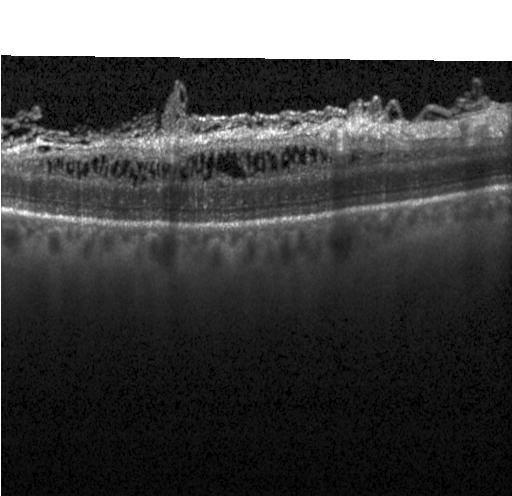 Retinal OCT cross-section.
Finding: DME.